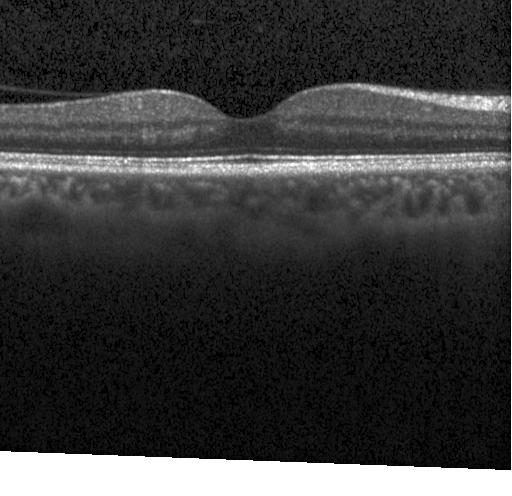 Impression: neither choroidal neovascularization, diabetic macular edema, nor drusen.